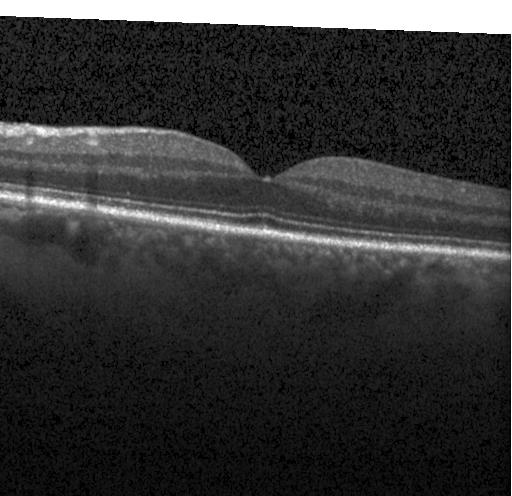 Retinal OCT B-scan · Heidelberg Spectralis OCT system · SD-OCT · macular scan.
Finding: no choroidal neovascularization, no diabetic macular edema, and no drusen.